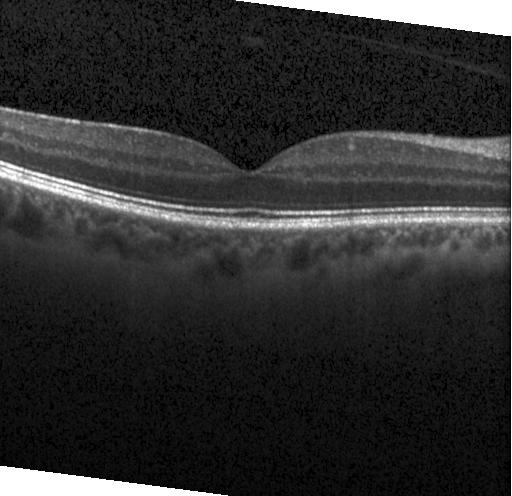
Heidelberg Spectralis OCT system; optical coherence tomography scan; spectral-domain optical coherence tomography.
Diagnosis: neither choroidal neovascularization, diabetic macular edema, nor drusen.